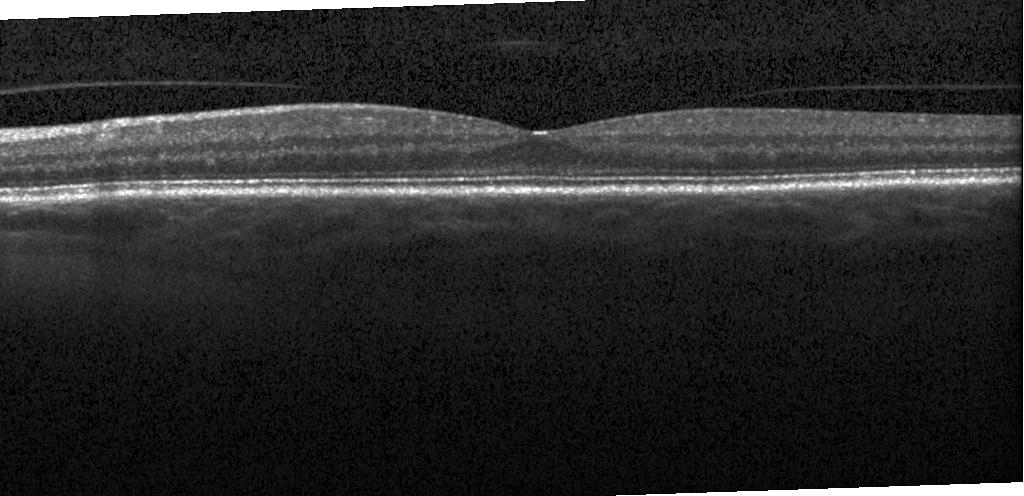
Impression: no CNV, no DME, and no drusen.